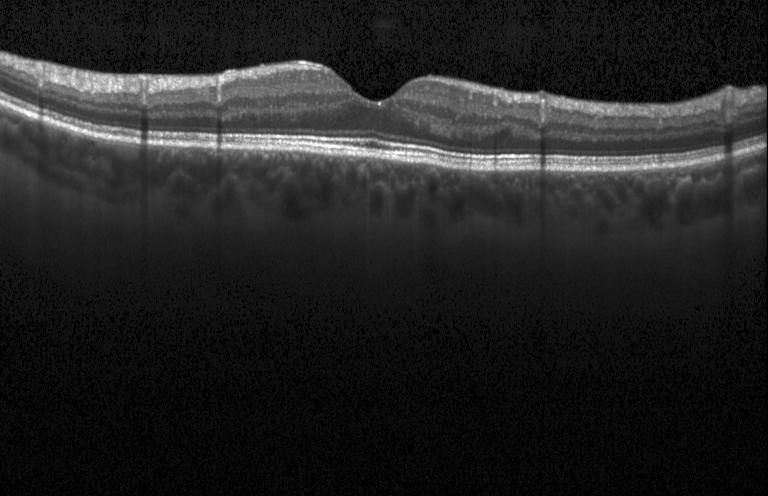

Macular OCT demonstrating no CNV, no DME, and no drusen.